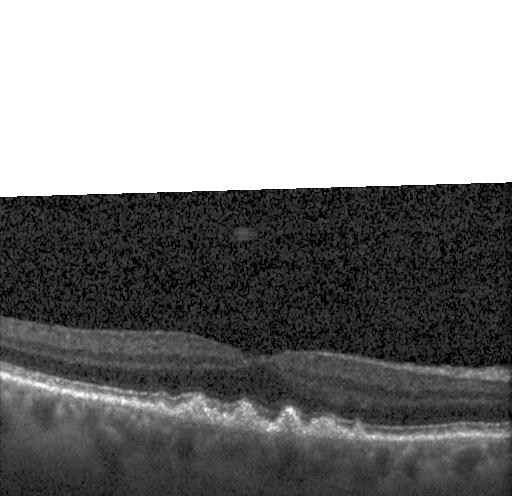

Heidelberg Spectralis. Spectral-domain optical coherence tomography. OCT line scan. Centered on the fovea — Dx: sub-RPE drusenoid deposits.